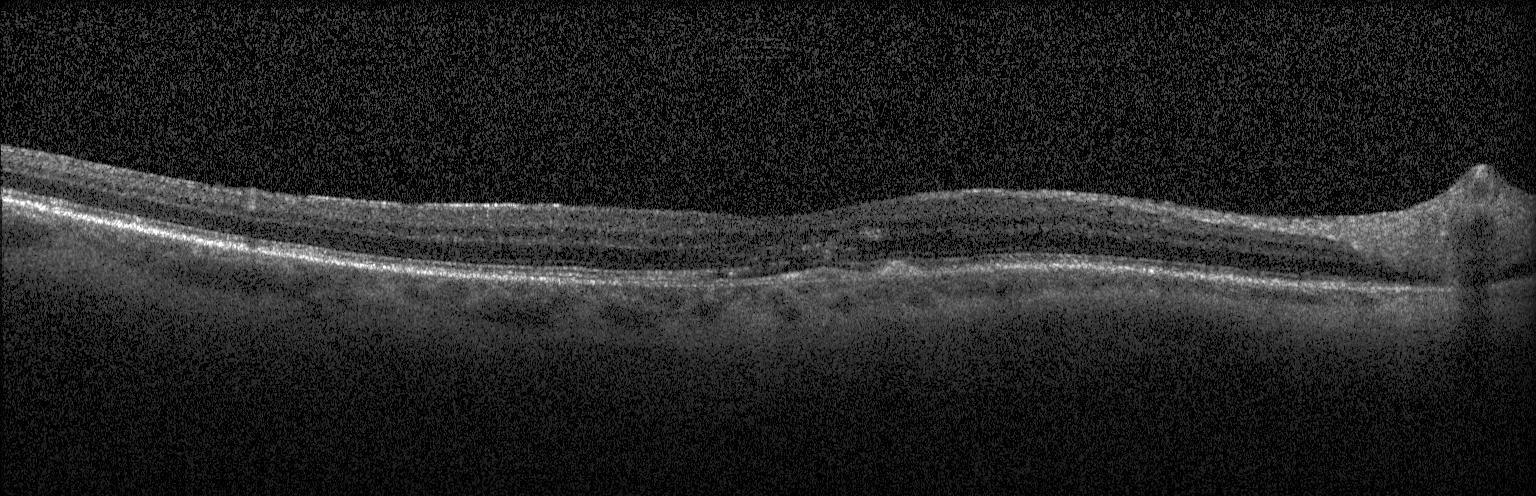
Finding: a choroidal neovascular membrane.